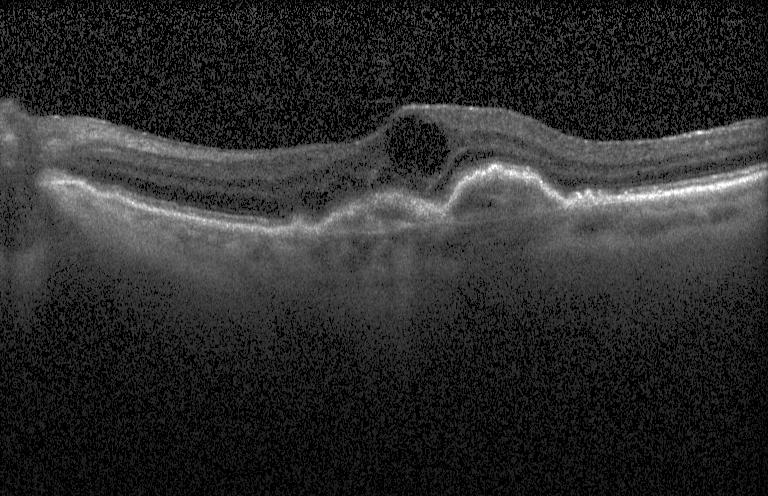

The scan shows a choroidal neovascular membrane.